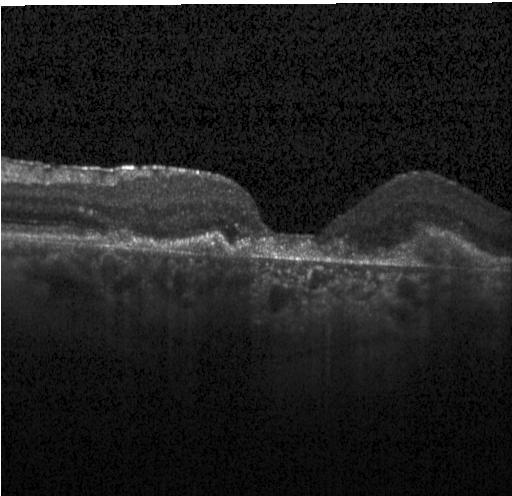
Choroidal neovascularization.